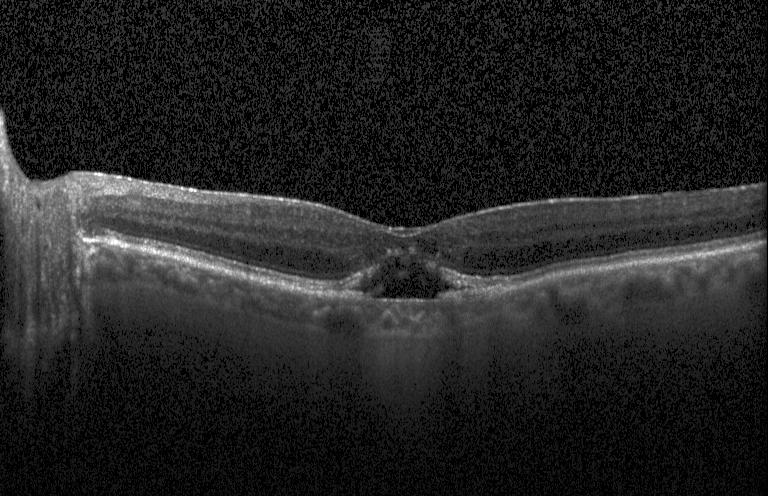 Through the macula; optical coherence tomography scan; SD-OCT.
Impression: a choroidal neovascular membrane.